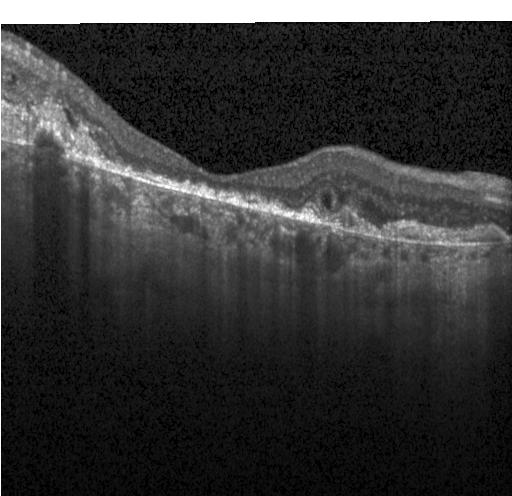 Finding: a choroidal neovascular membrane.